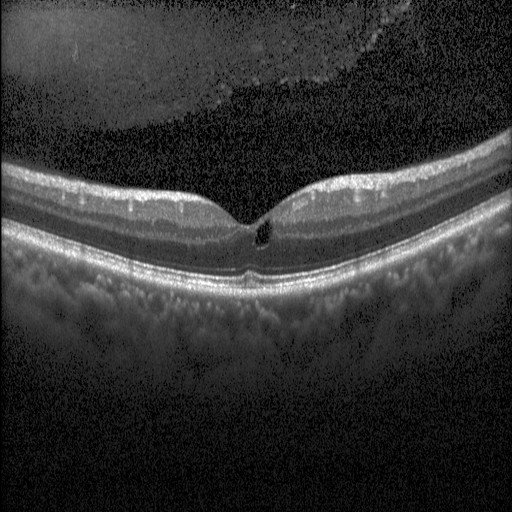
Retinal OCT B-scan — OCT finding: DME.